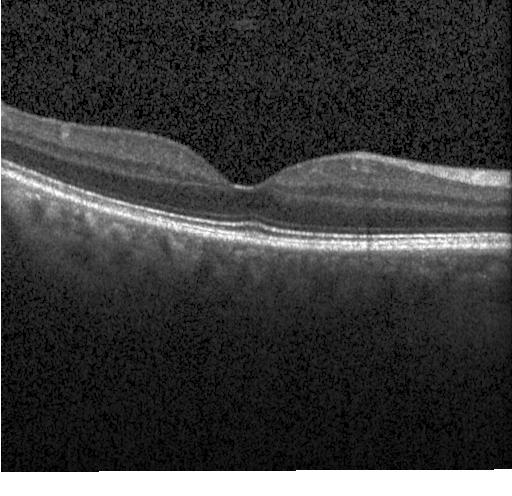

Finding: no choroidal neovascularization, no diabetic macular edema, and no drusen.